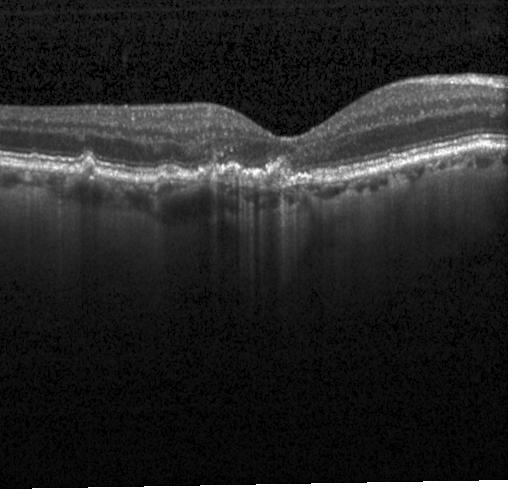 Dx: a choroidal neovascular membrane.